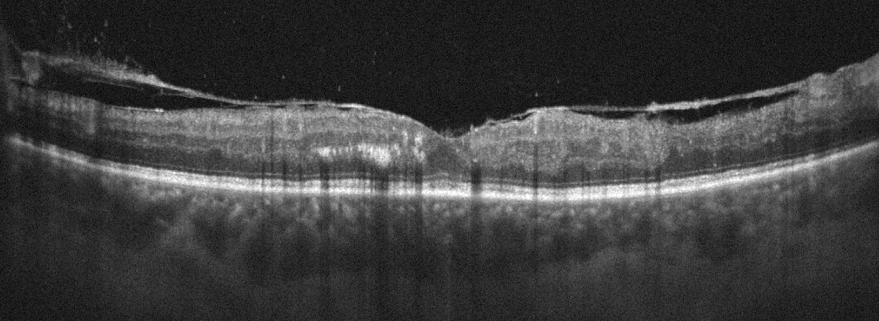 OCT B-scan, acquired on an Optovue Avanti RTVue XR, fovea-centered
Diagnosis: diabetic macular edema (DME).